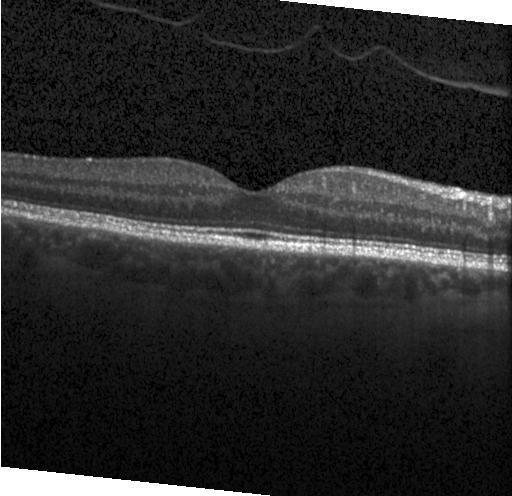

Fovea-centered · Heidelberg Spectralis · retinal OCT cross-section · SD-OCT. Impression: neither CNV, DME, nor drusen.